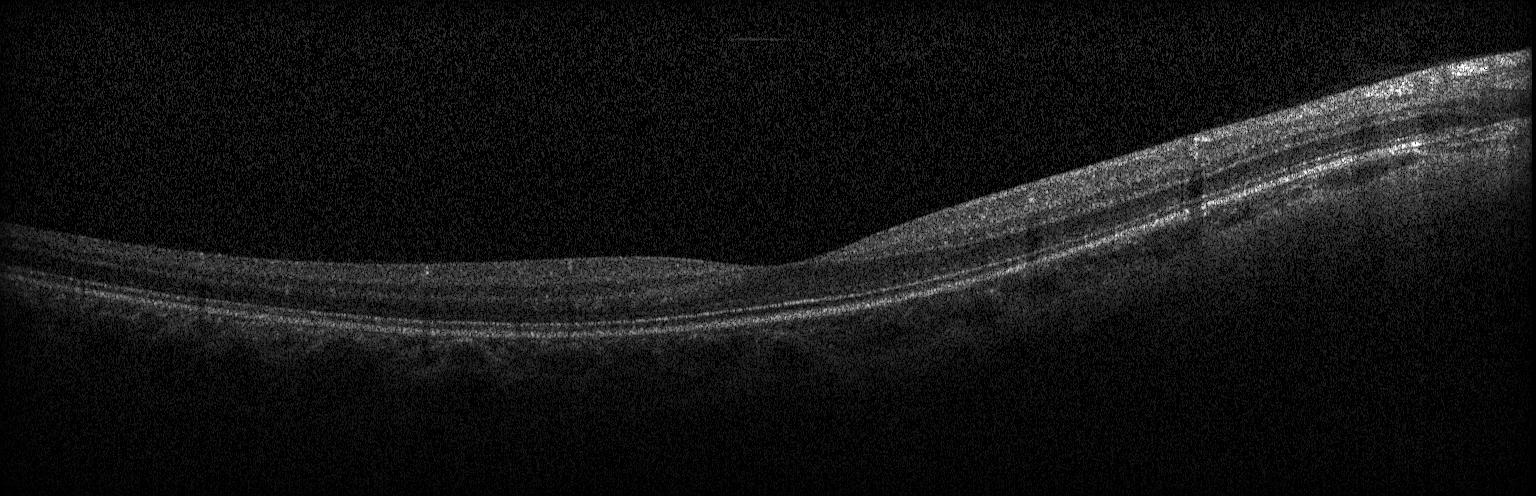
Optical coherence tomography scan; Heidelberg Spectralis; spectral-domain OCT; macular scan — Impression: no evidence of choroidal neovascularization, diabetic macular edema, or drusen.